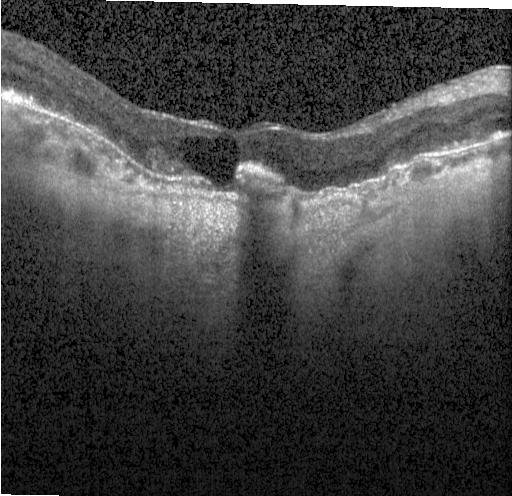

Spectral-domain optical coherence tomography; retinal OCT cross-section; horizontal scan through the fovea. A choroidal neovascular membrane.